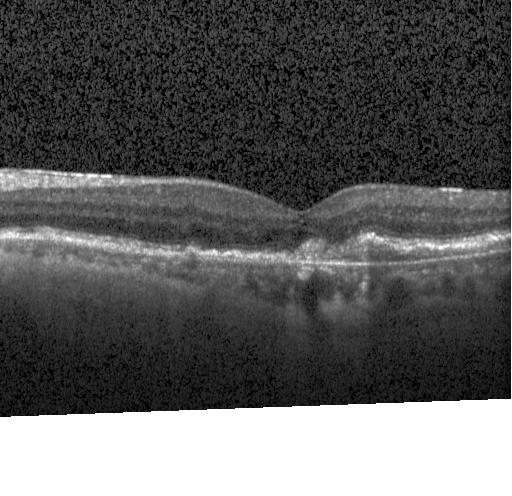
Spectral-domain OCT B-scan: choroidal neovascularization.